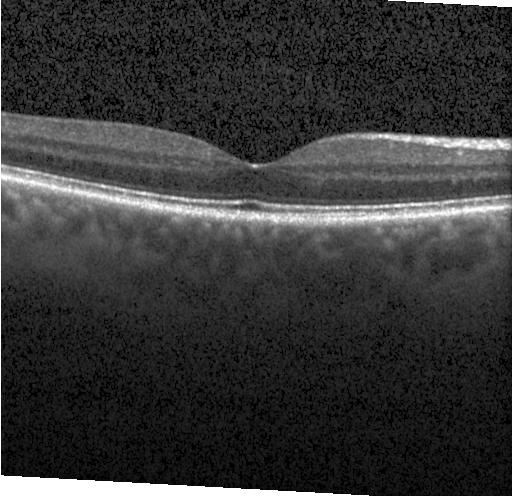 Spectral-domain optical coherence tomography; optical coherence tomography B-scan. Dx: no CNV, no DME, and no drusen.